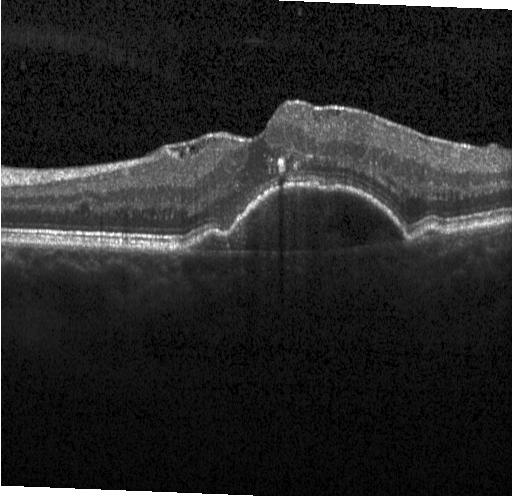

OCT B-scan showing choroidal neovascularization (CNV).